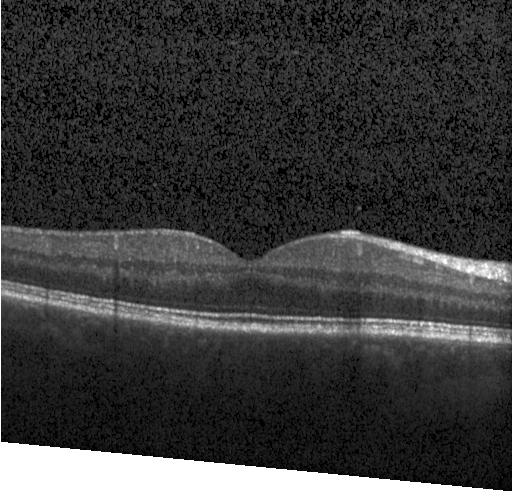 Optical coherence tomography scan · SD-OCT
Macular OCT: no CNV, DME, or drusen.